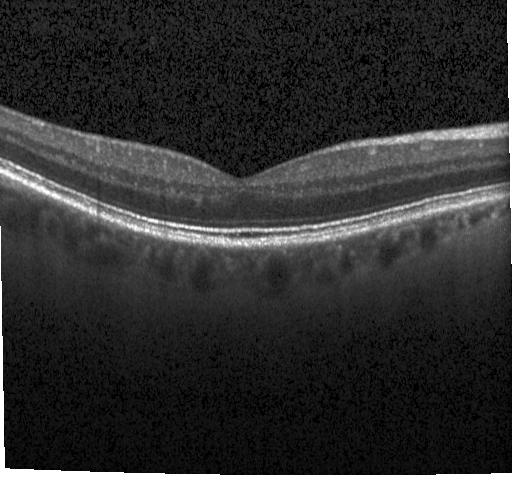
Macular scan, optical coherence tomography B-scan, instrument: Heidelberg Spectralis
This B-scan demonstrates no evidence of choroidal neovascularization, diabetic macular edema, or drusen.